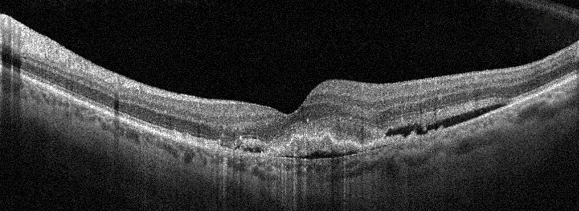
Optical coherence tomography scan; OS
Diagnosis: age-related macular degeneration.